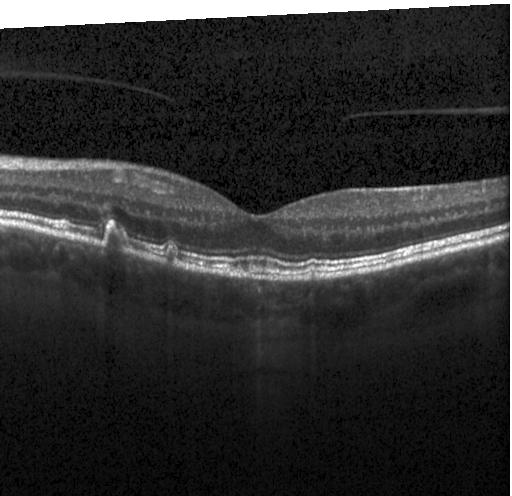
OCT scan showing multiple drusen.